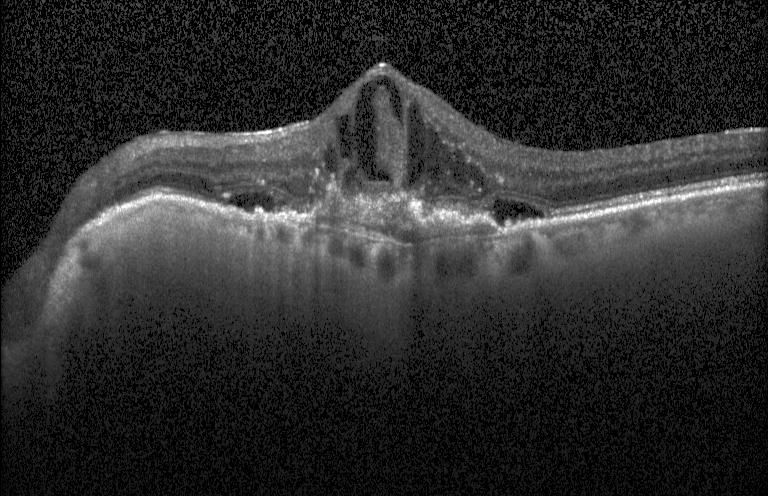 Heidelberg Spectralis OCT system, optical coherence tomography B-scan, spectral-domain optical coherence tomography — Impression: choroidal neovascularization.